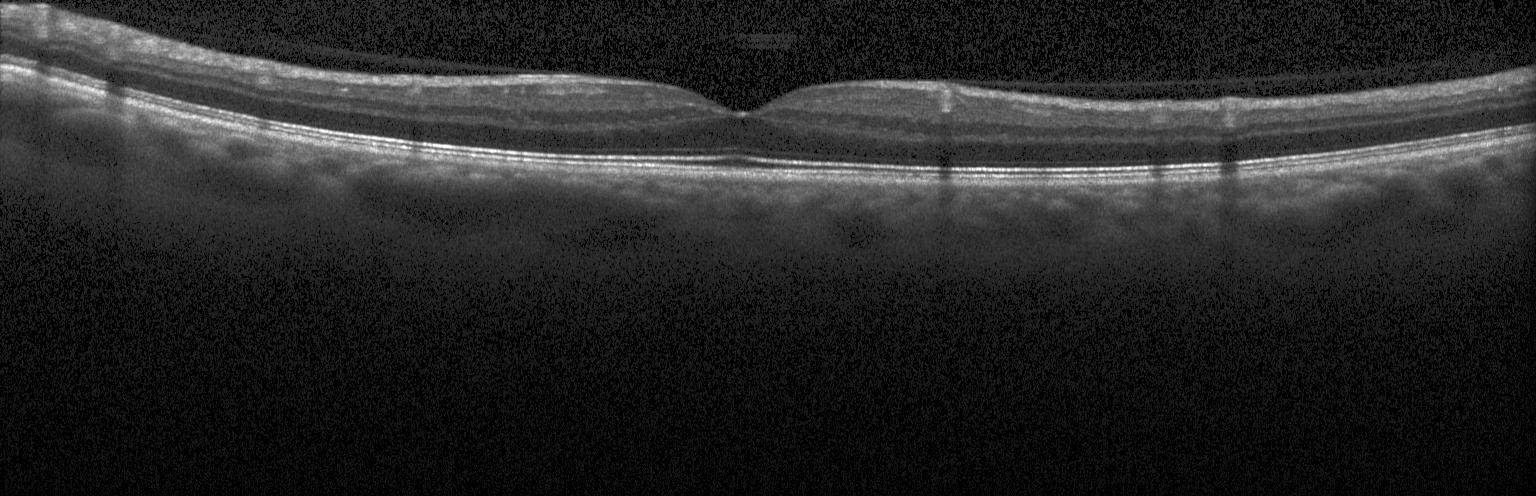 Finding: no evidence of CNV, DME, or drusen.